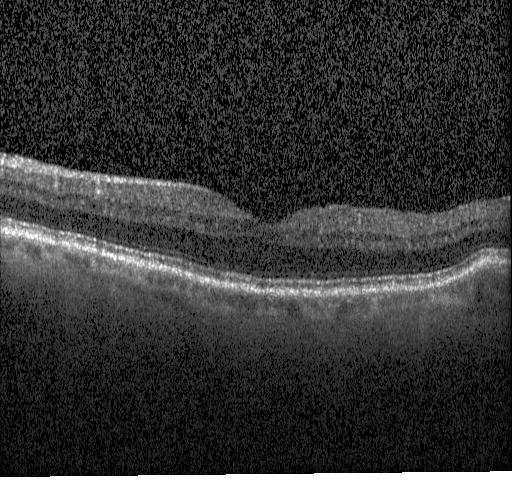

Instrument: Heidelberg Spectralis; OCT line scan; spectral-domain optical coherence tomography. Diagnosis: no CNV, DME, or drusen.